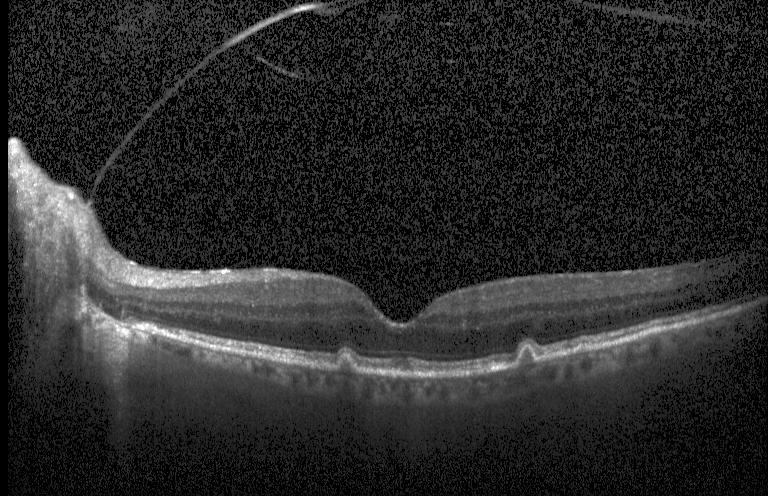 Macular OCT demonstrating multiple drusen.